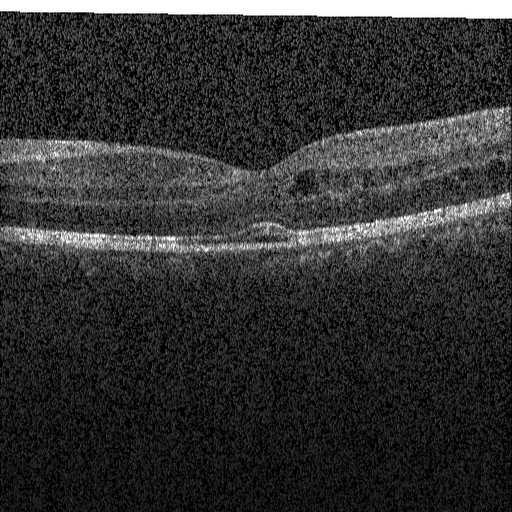

Retinal OCT B-scan, through the macula, spectral-domain optical coherence tomography, Heidelberg Spectralis OCT system — This B-scan demonstrates diabetic macular edema.